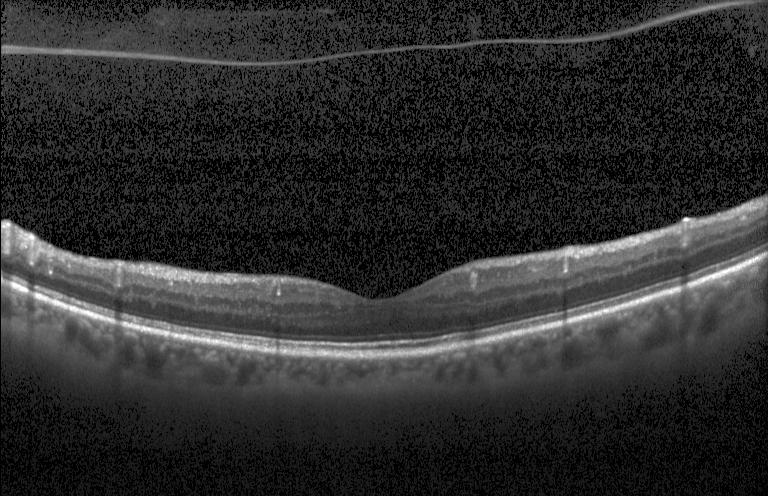 Through the macula · SD-OCT · retinal OCT B-scan
Impression: no CNV, no DME, and no drusen.